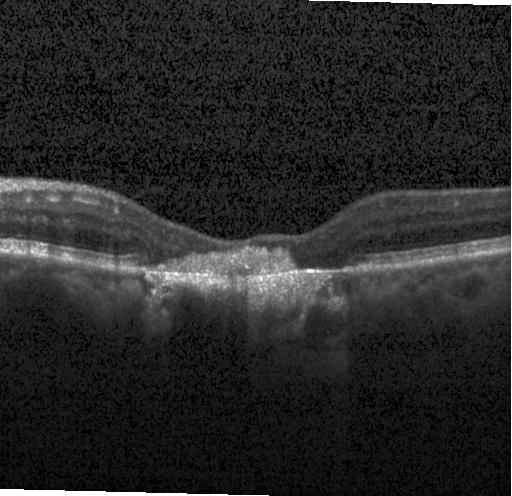
Diagnosis: a choroidal neovascular membrane.